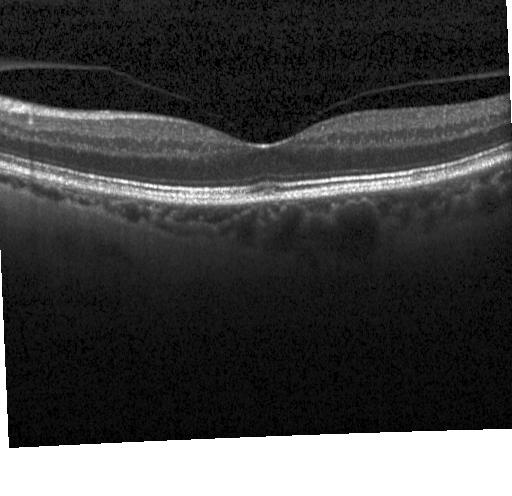
OCT scan showing no evidence of CNV, DME, or drusen.